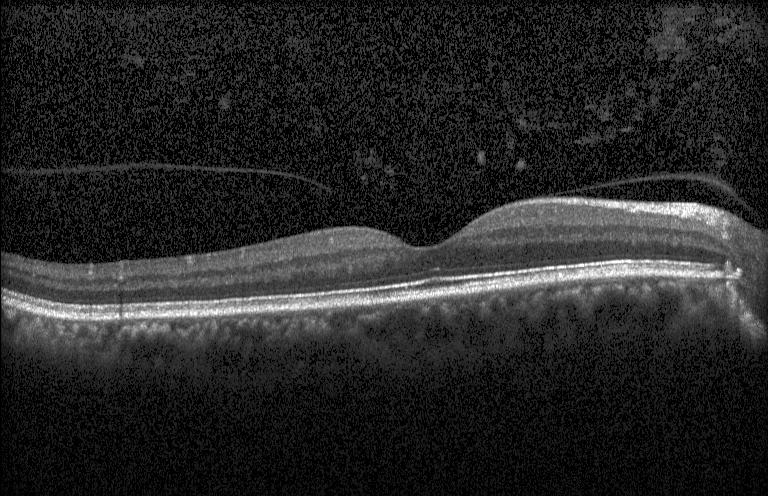 Acquired on a Heidelberg Spectralis · horizontal scan through the fovea · optical coherence tomography scan
Assessment: no choroidal neovascularization, diabetic macular edema, or drusen.